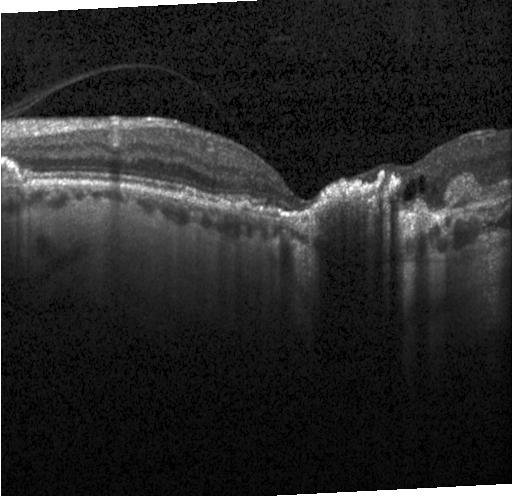

Through the macula, SD-OCT, acquired on a Heidelberg Spectralis, optical coherence tomography B-scan — Finding: choroidal neovascularization.